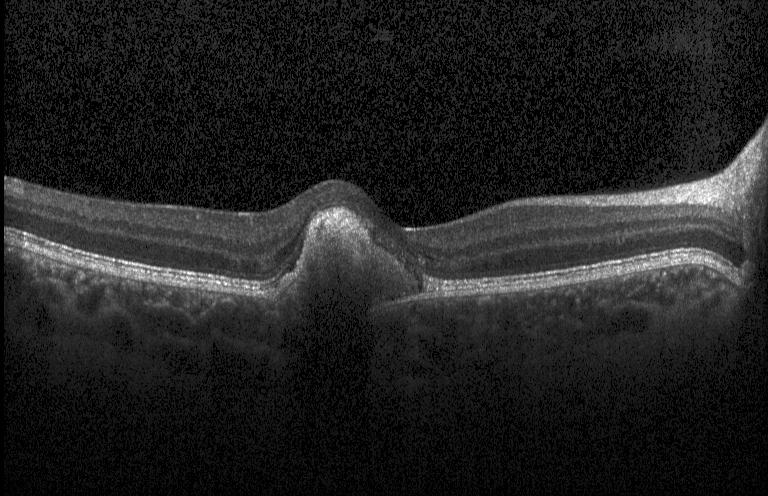 OCT finding: a choroidal neovascular membrane.